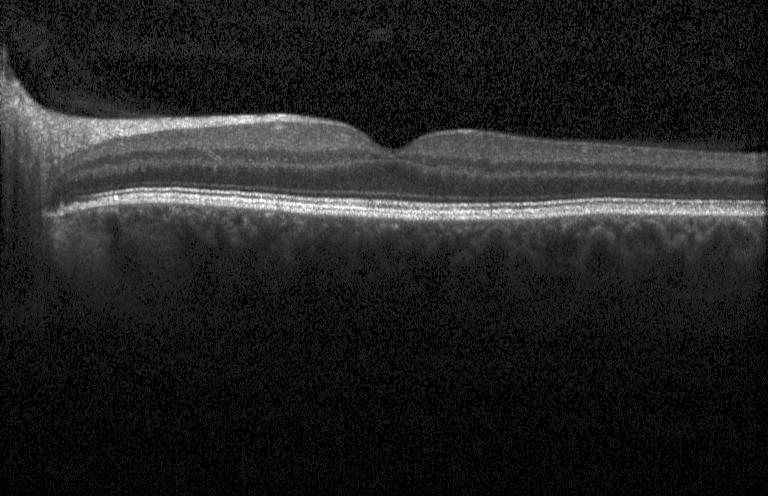

OCT line scan, instrument: Heidelberg Spectralis, SD-OCT. Impression: no choroidal neovascularization, no diabetic macular edema, and no drusen.